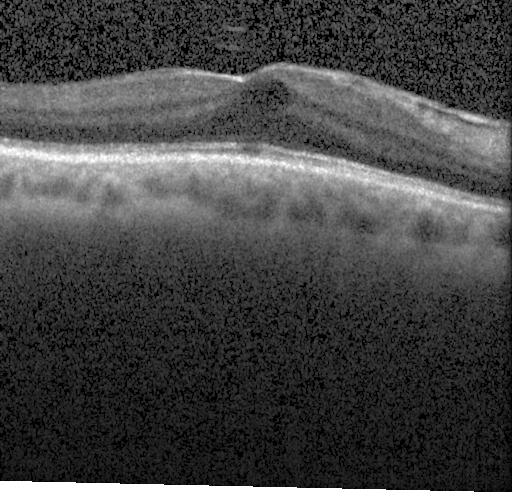 Retinal OCT cross-section. Macular OCT: diabetic macular edema (DME).